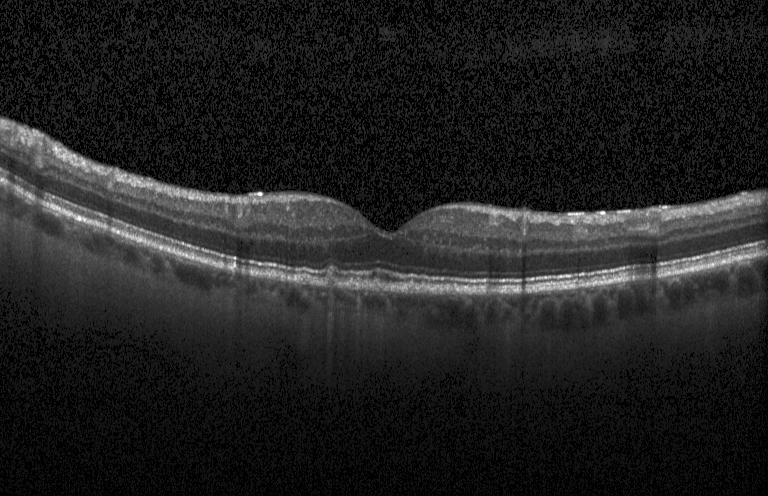

Macular OCT: drusen.